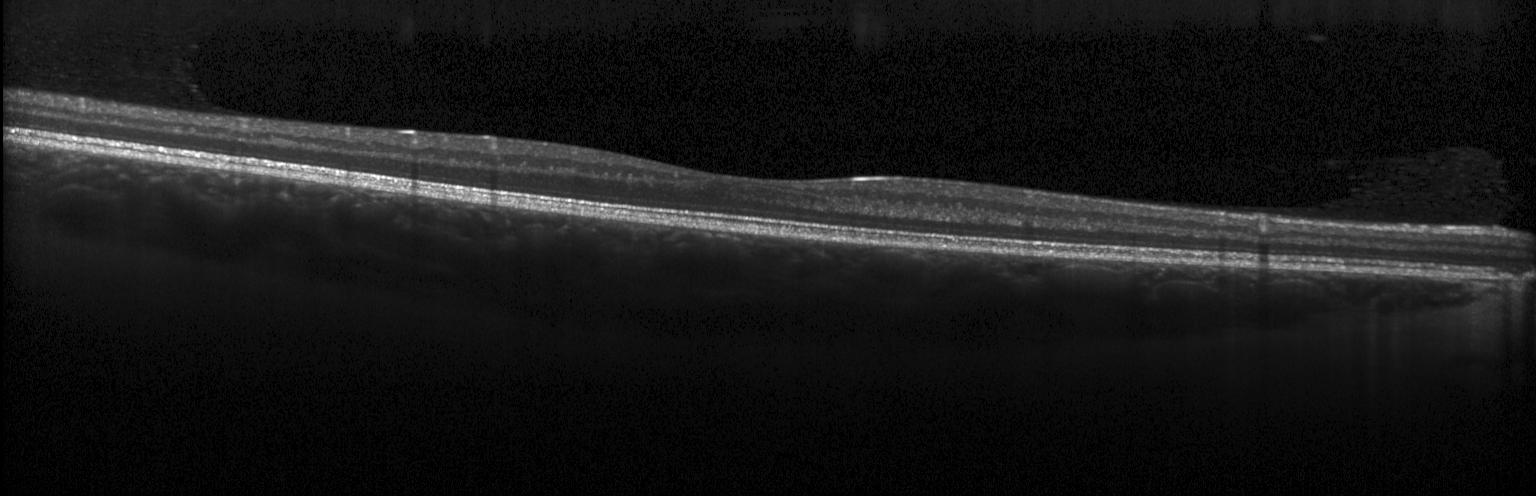
Macular OCT demonstrating no choroidal neovascularization, no diabetic macular edema, and no drusen.